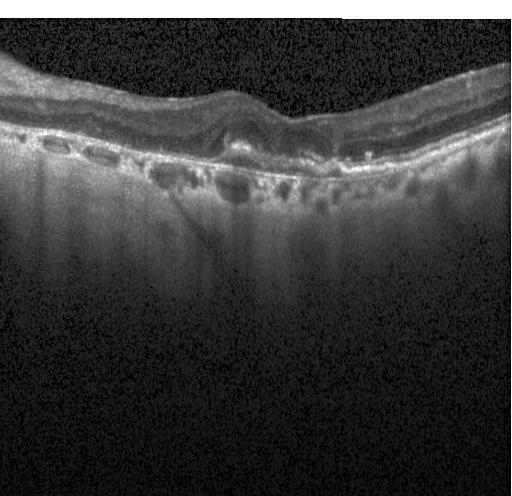
Optical coherence tomography scan · spectral-domain OCT.
The scan shows a choroidal neovascular membrane.